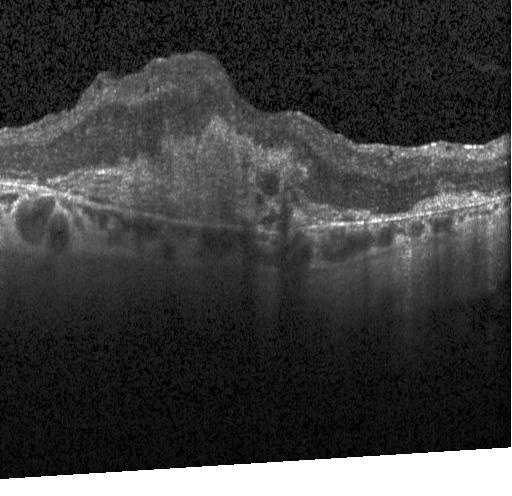
Finding: choroidal neovascularization (CNV).